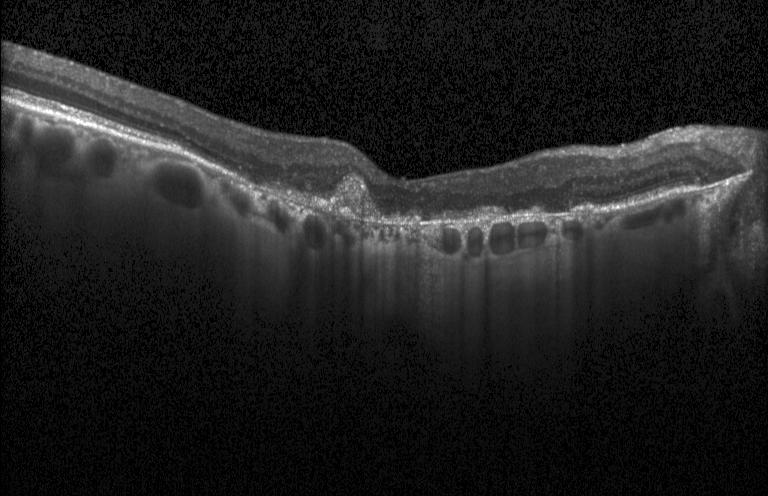
Macular scan · OCT B-scan — Dx: choroidal neovascularization.